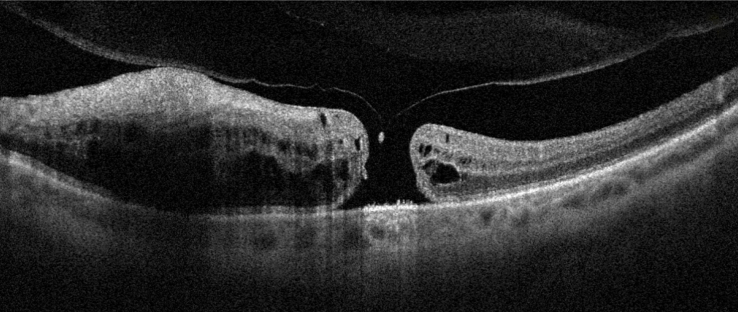 Fovea-centered, OCT line scan.
Diagnosis: VID.